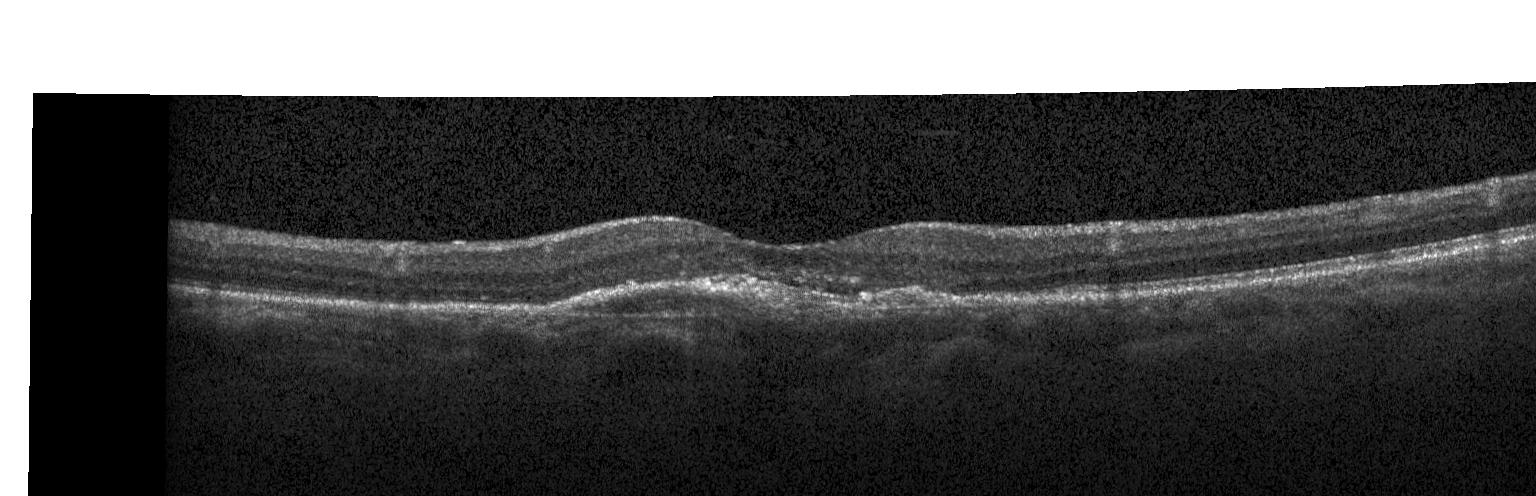 Finding: CNV.